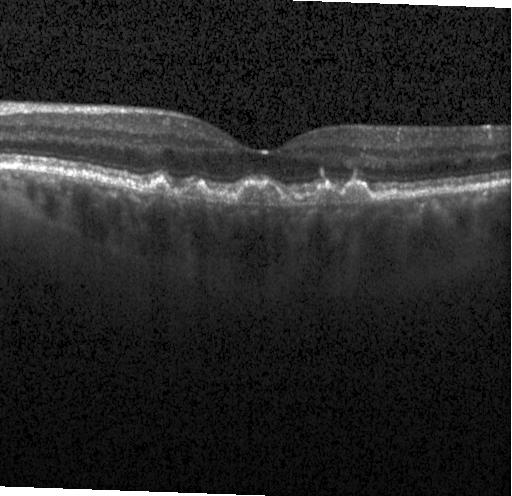 Macular OCT: sub-RPE drusenoid deposits.